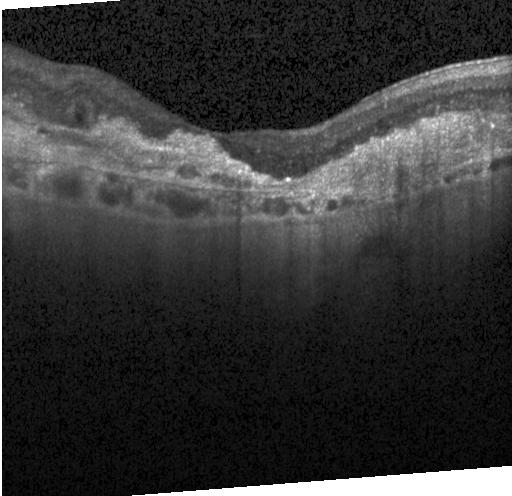
Finding: choroidal neovascularization.